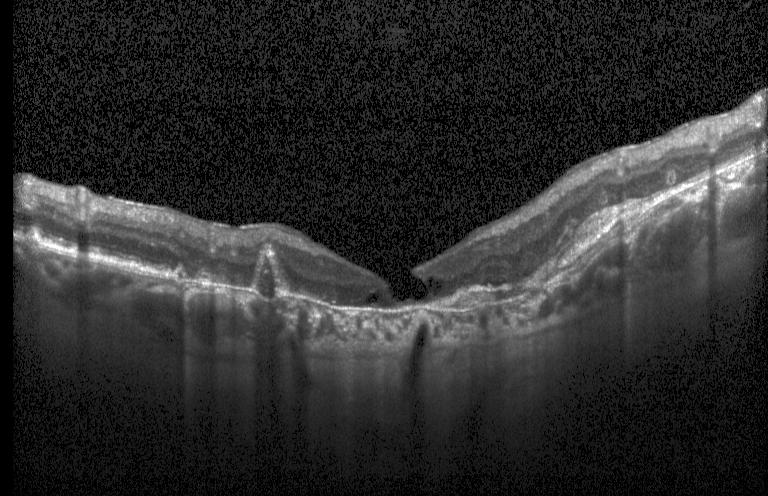 Impression: choroidal neovascularization.